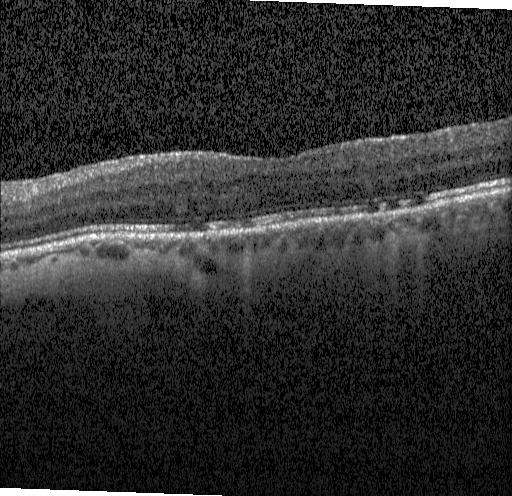
Macular scan, retinal OCT B-scan, spectral-domain OCT
Impression: no choroidal neovascularization, diabetic macular edema, or drusen.